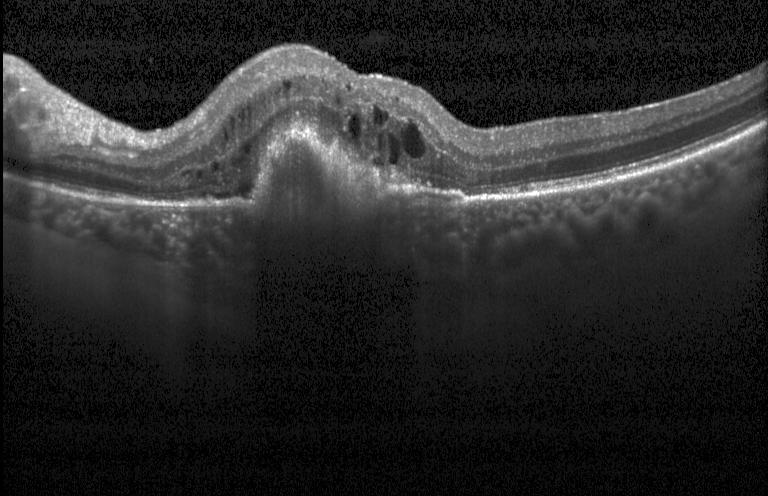

Macular OCT demonstrating choroidal neovascularization.